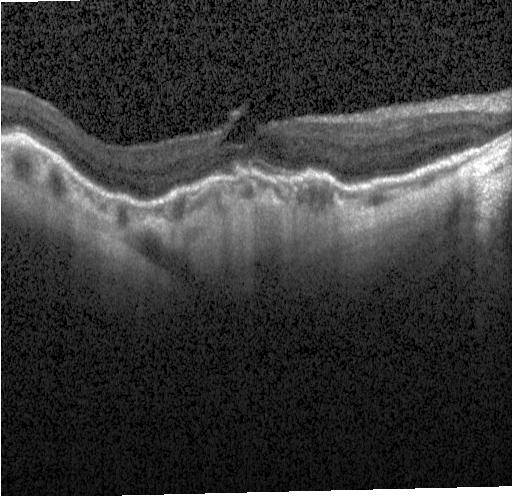

Acquired on a Heidelberg Spectralis; horizontal scan through the fovea; OCT line scan
Impression: a choroidal neovascular membrane.